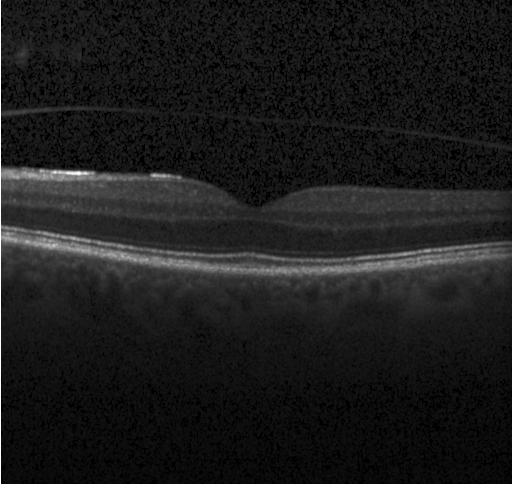
Macular OCT demonstrating no choroidal neovascularization, no diabetic macular edema, and no drusen.